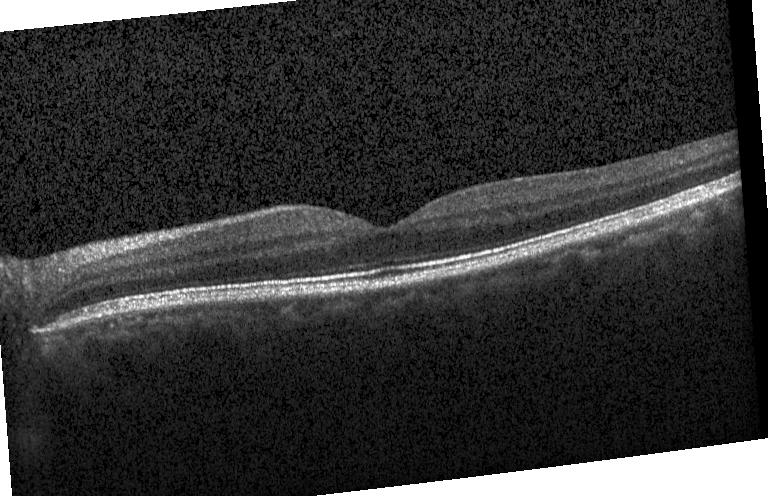

OCT scan showing no evidence of CNV, DME, or drusen.